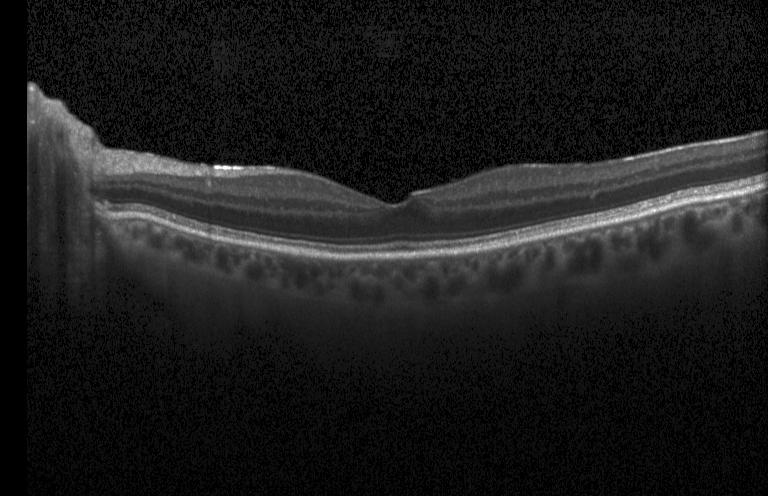
Diagnosis: no choroidal neovascularization, no diabetic macular edema, and no drusen.